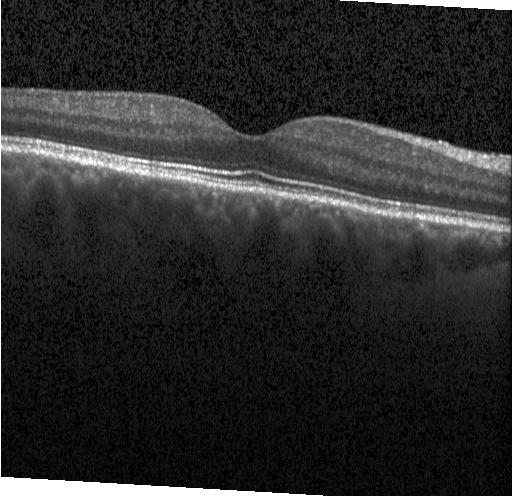
Optical coherence tomography scan, macular scan — The scan shows no choroidal neovascularization, no diabetic macular edema, and no drusen.